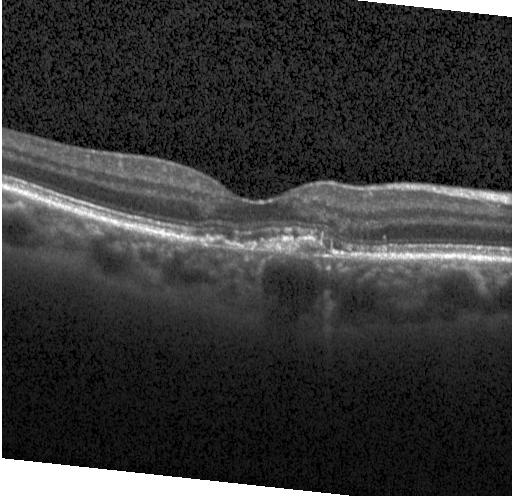

Dx: CNV.